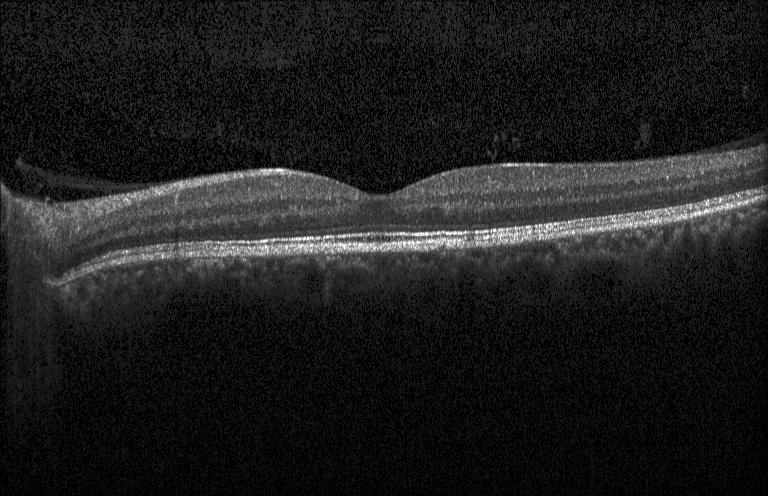

Dx: no evidence of choroidal neovascularization, diabetic macular edema, or drusen.